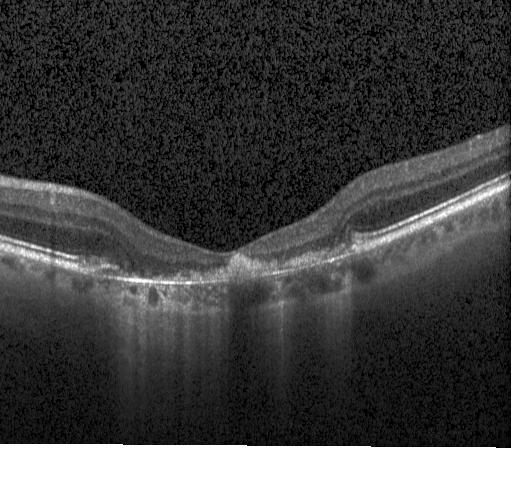
Optical coherence tomography scan — Impression: a choroidal neovascular membrane.